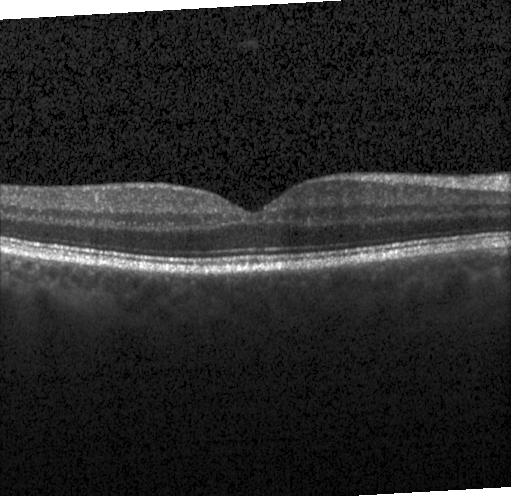

OCT line scan.
No CNV, DME, or drusen.